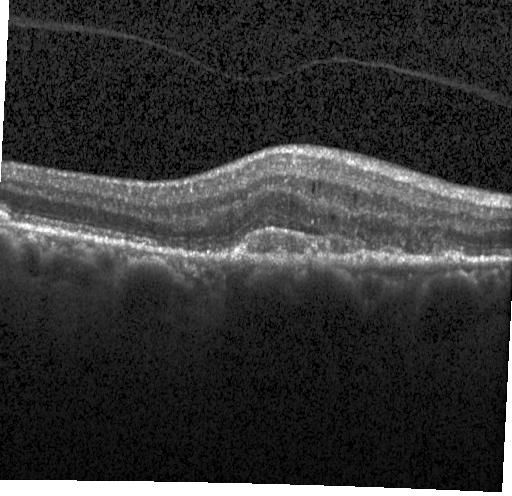

Macular OCT demonstrating choroidal neovascularization (CNV).